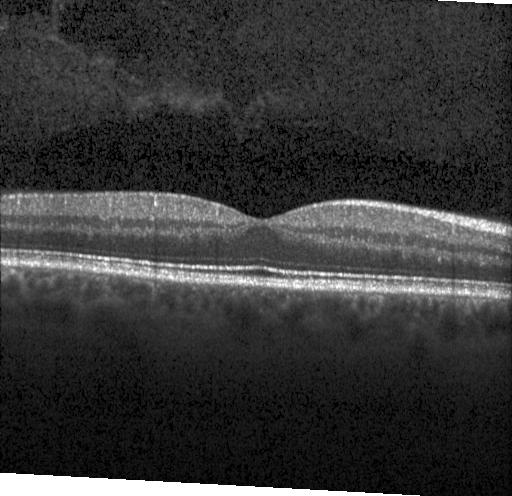 Heidelberg Spectralis · macular scan · optical coherence tomography scan · SD-OCT
The scan shows no evidence of CNV, DME, or drusen.